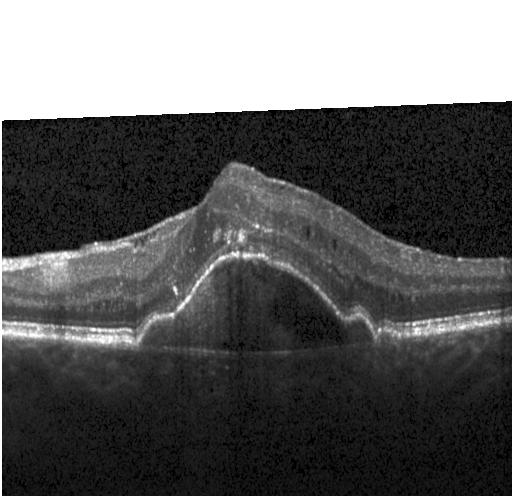

Heidelberg Spectralis OCT system · retinal OCT B-scan · macular scan · spectral-domain OCT. Impression: a choroidal neovascular membrane.